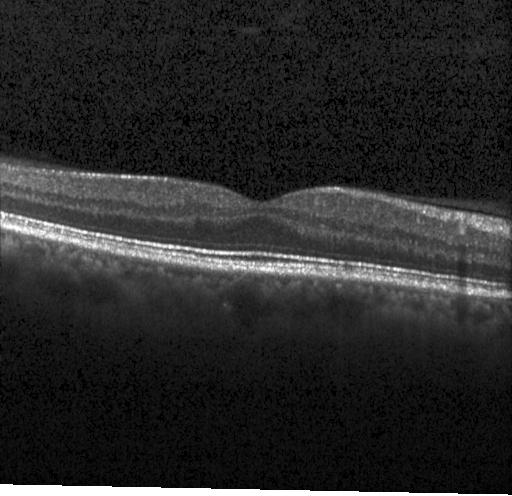 Optical coherence tomography B-scan. Finding: no choroidal neovascularization, no diabetic macular edema, and no drusen.